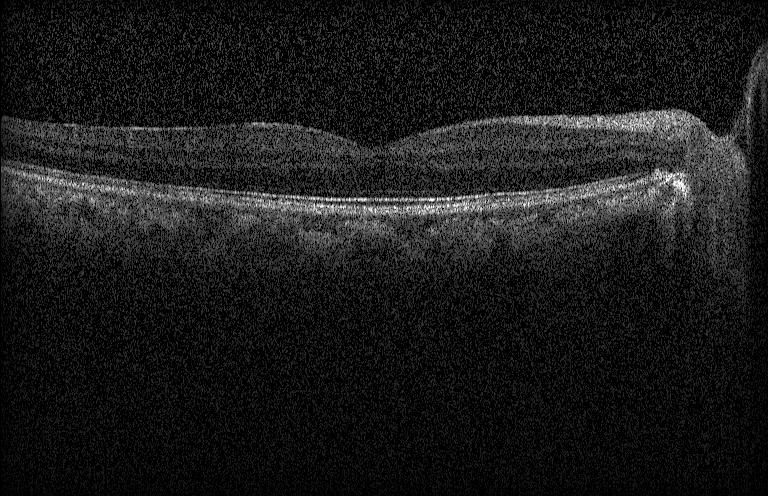 Acquired on a Heidelberg Spectralis, centered on the fovea, retinal OCT B-scan — Diagnosis: no CNV, DME, or drusen.